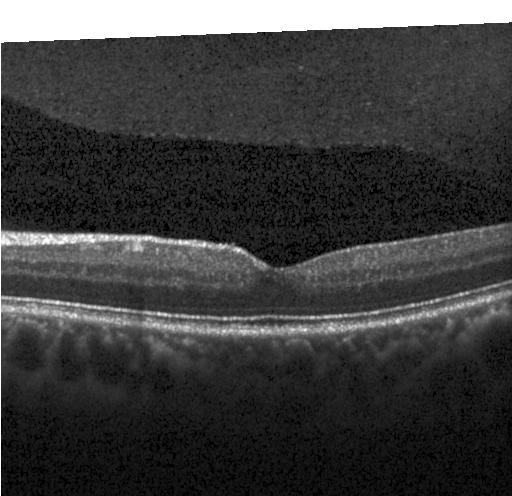
Fovea-centered. Optical coherence tomography scan. Spectral-domain OCT
The scan shows no choroidal neovascularization, diabetic macular edema, or drusen.